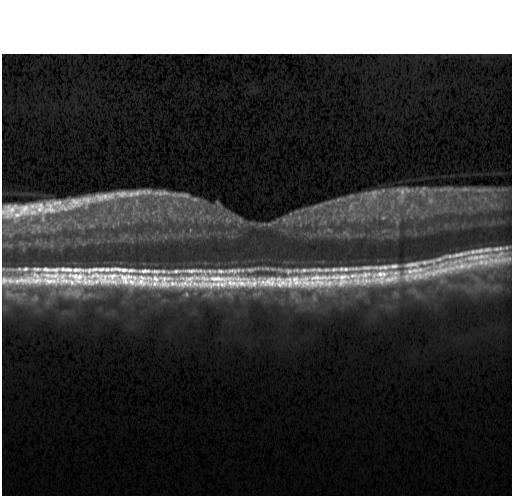
OCT B-scan. SD-OCT. Heidelberg Spectralis — Finding: neither choroidal neovascularization, diabetic macular edema, nor drusen.